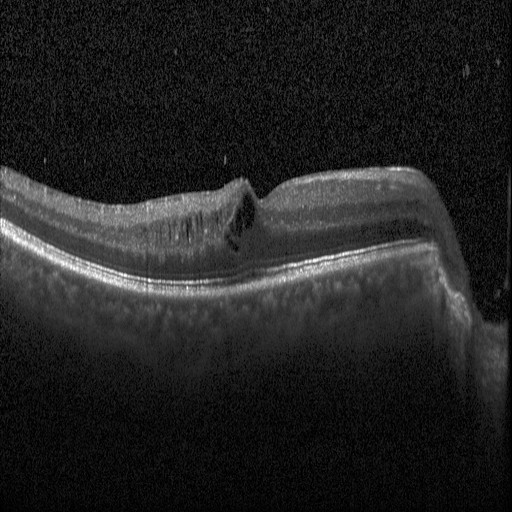

Retinal OCT cross-section showing diabetic macular edema.